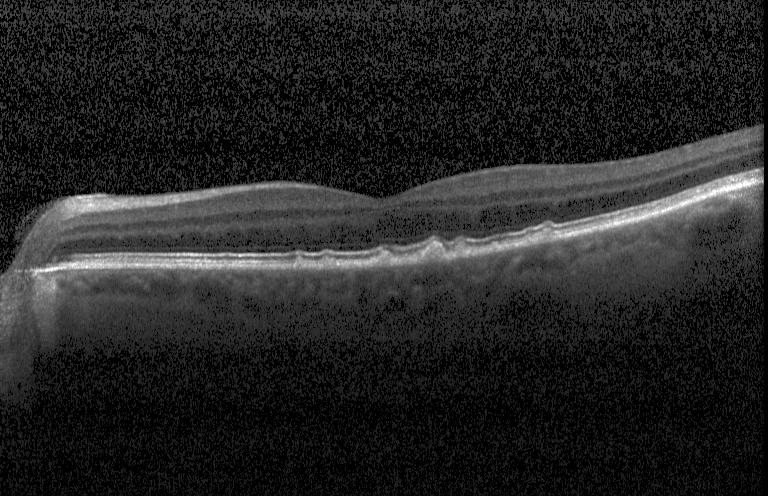
Finding: drusen.